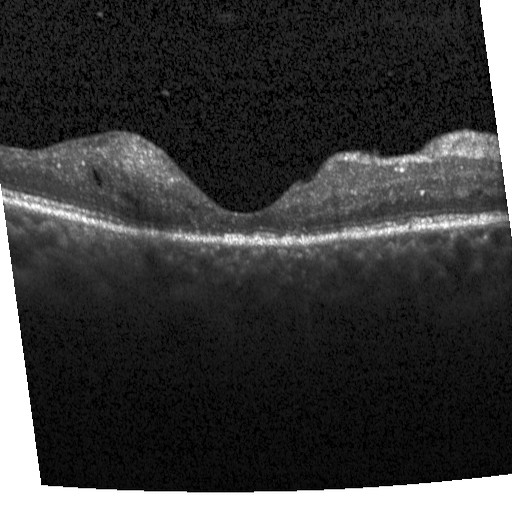
Diabetic macular edema (DME).